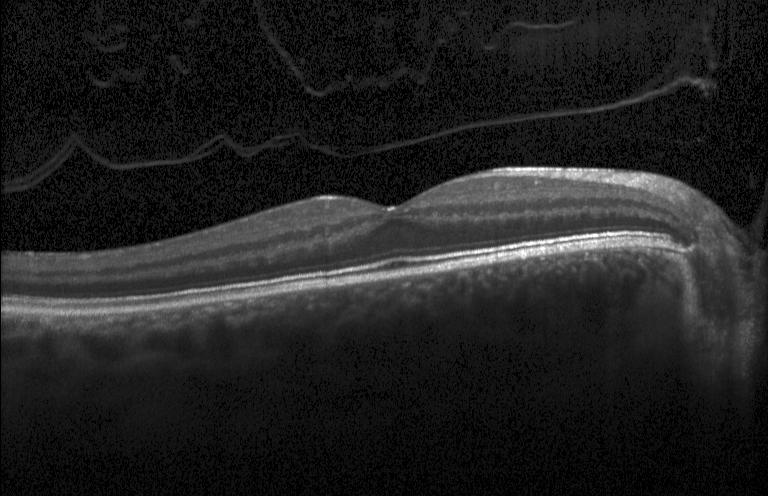
Retinal OCT cross-section — Finding: no evidence of CNV, DME, or drusen.